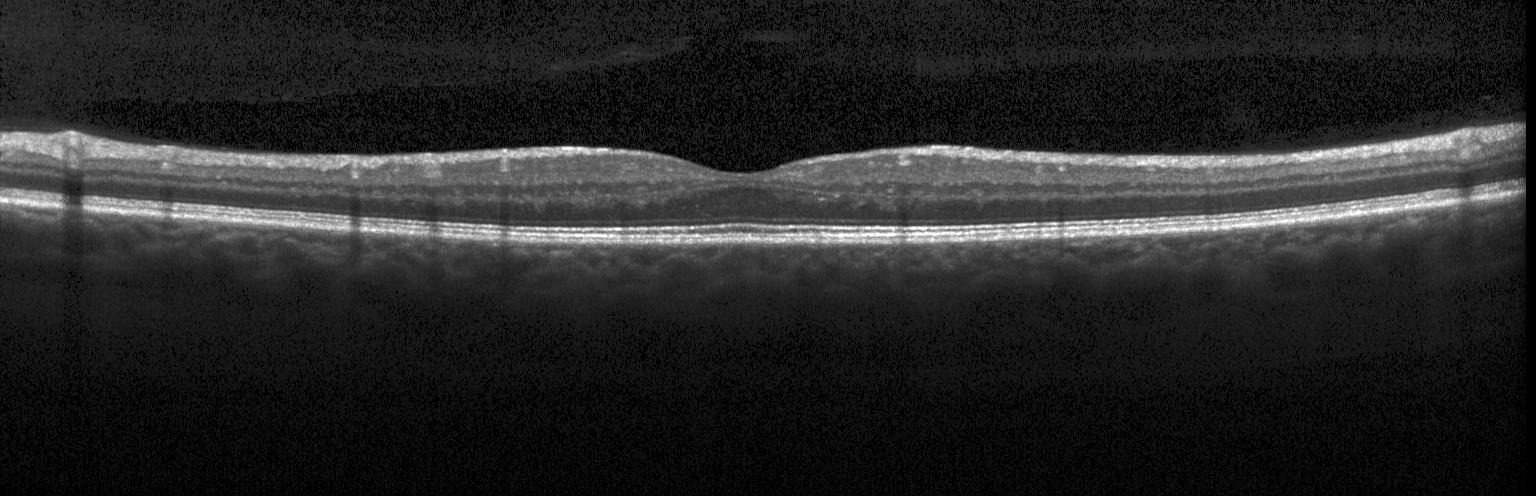 Diagnosis: neither choroidal neovascularization, diabetic macular edema, nor drusen.